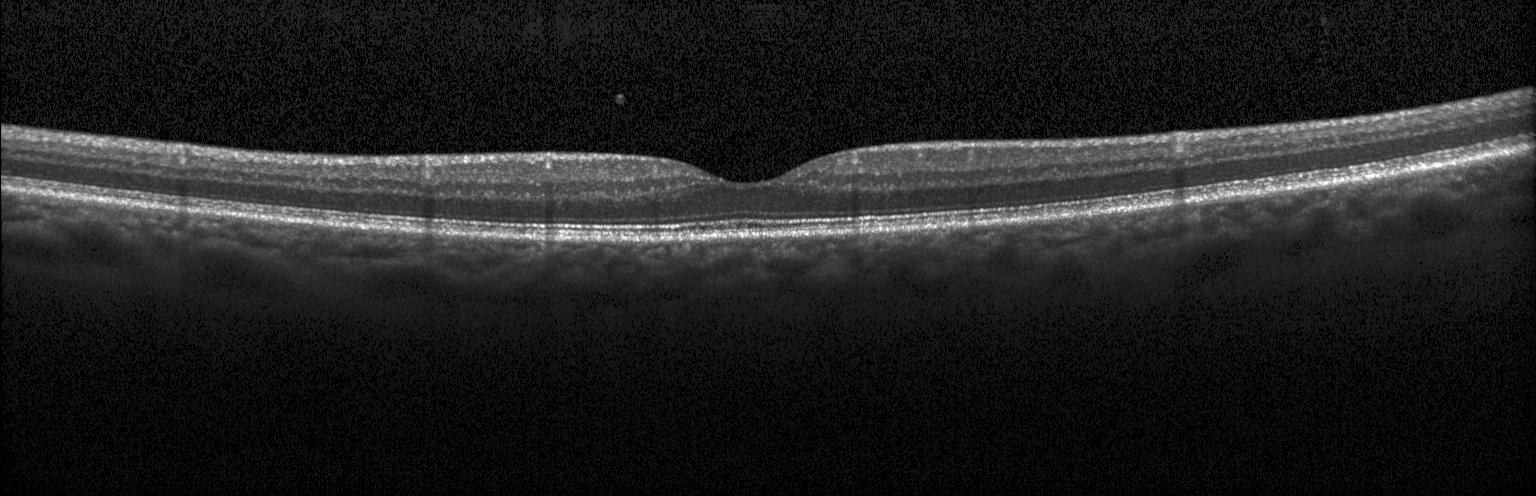
OCT B-scan; SD-OCT; Heidelberg Spectralis OCT system — OCT finding: neither choroidal neovascularization, diabetic macular edema, nor drusen.